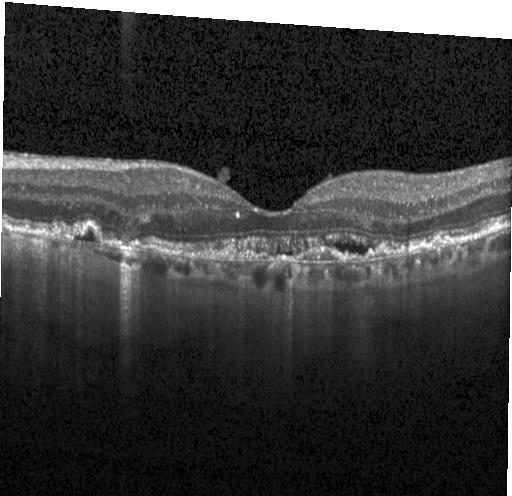 Instrument: Heidelberg Spectralis · fovea-centered · retinal OCT cross-section
Assessment: CNV.